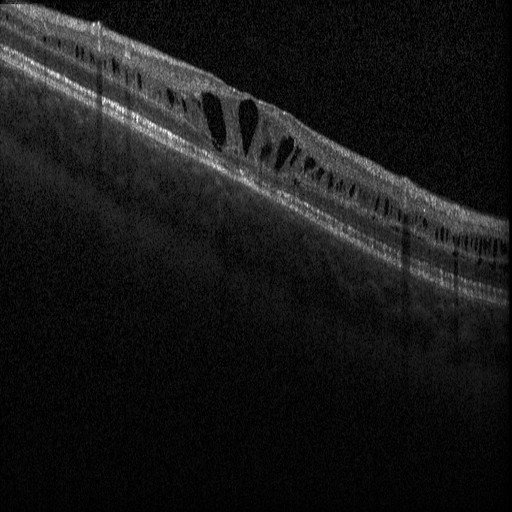

Through the macula, retinal OCT cross-section, SD-OCT. This B-scan demonstrates diabetic macular edema (DME).